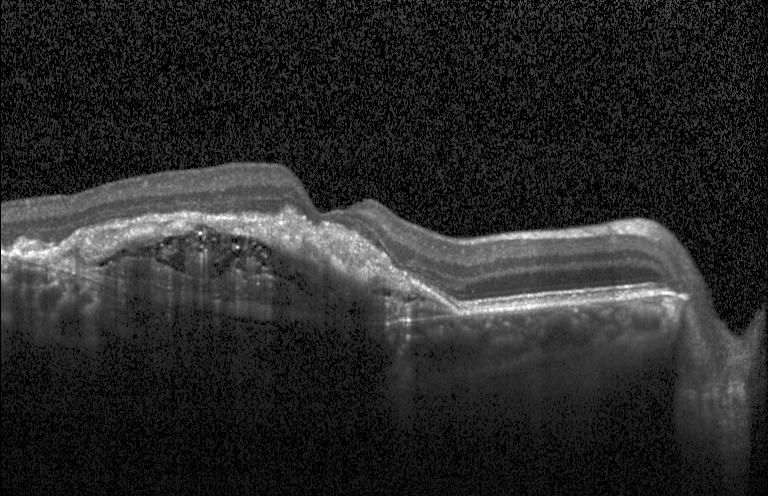 Retinal OCT B-scan. SD-OCT
Impression: choroidal neovascularization (CNV).